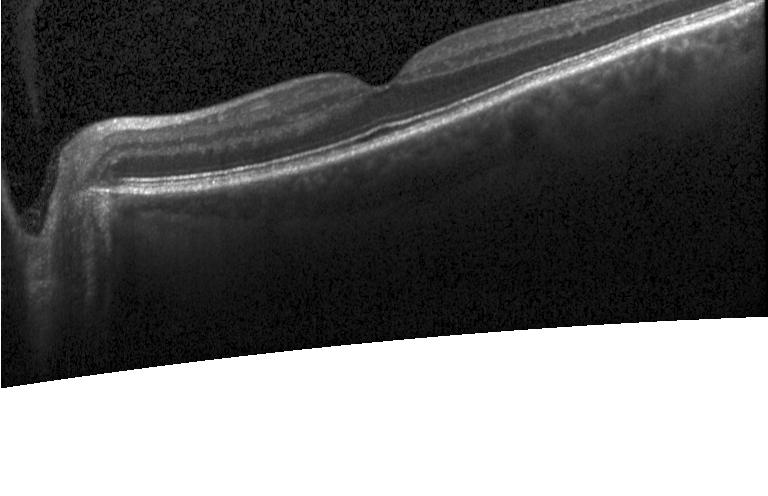 Retinal OCT B-scan.
OCT finding: no evidence of CNV, DME, or drusen.